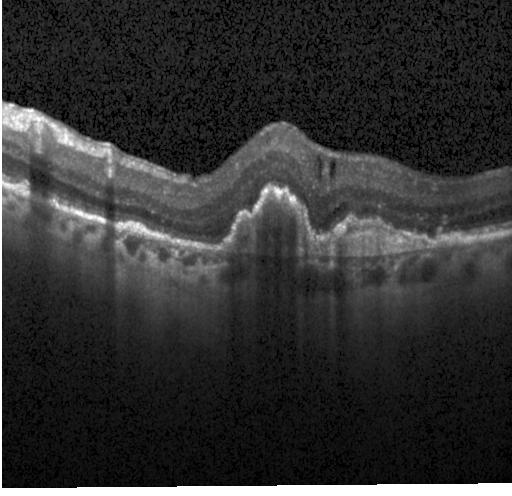

Finding: choroidal neovascularization.